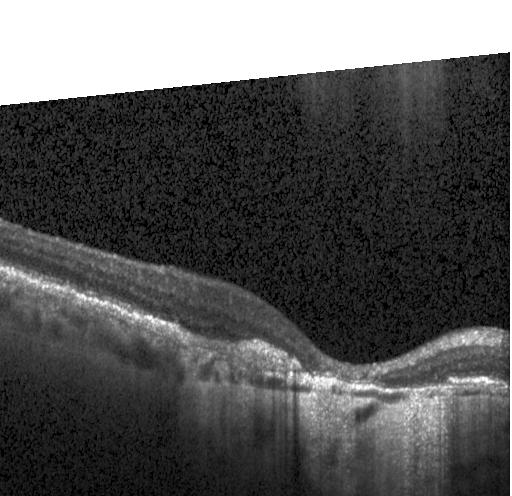

Acquired on a Heidelberg Spectralis · OCT B-scan — The scan shows CNV.